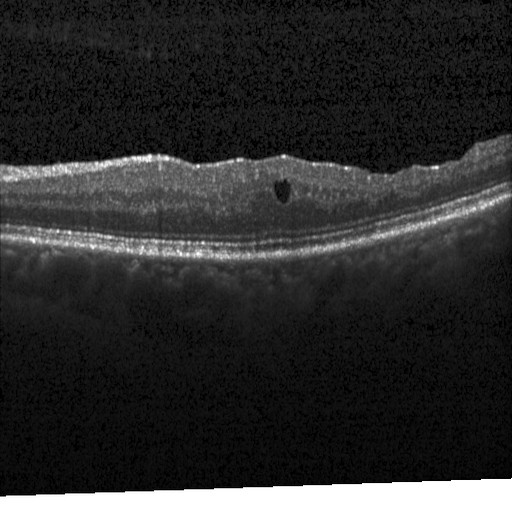
Finding: diabetic macular edema.